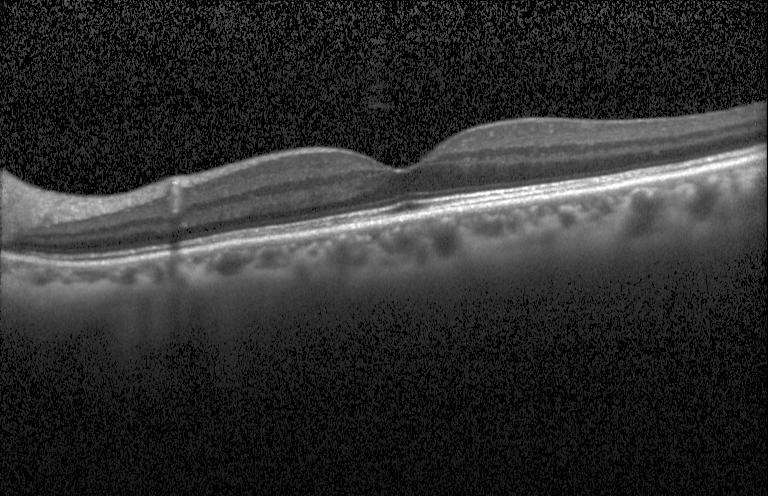
OCT B-scan showing no evidence of CNV, DME, or drusen.